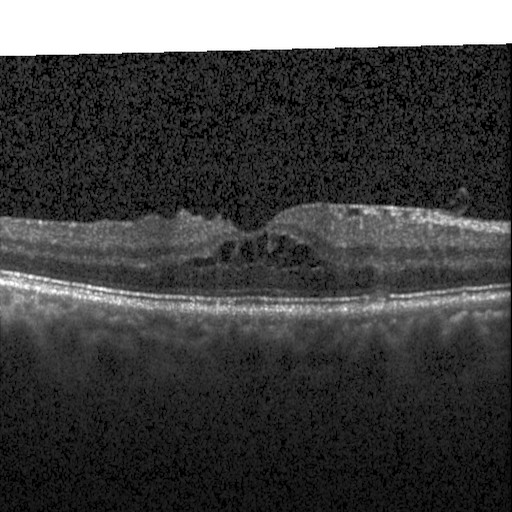 Dx: diabetic macular edema (DME).